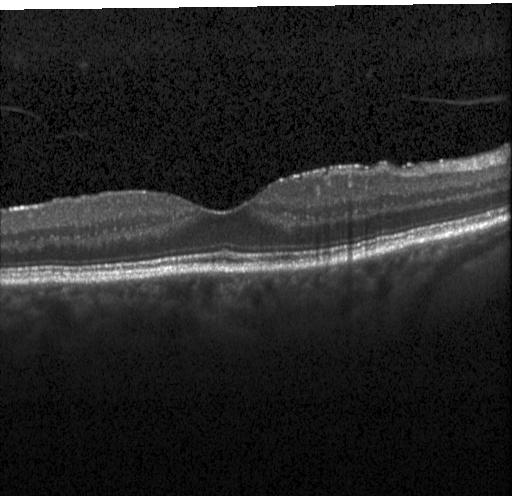
Retinal OCT B-scan · spectral-domain OCT · fovea-centered. Assessment: no evidence of choroidal neovascularization, diabetic macular edema, or drusen.